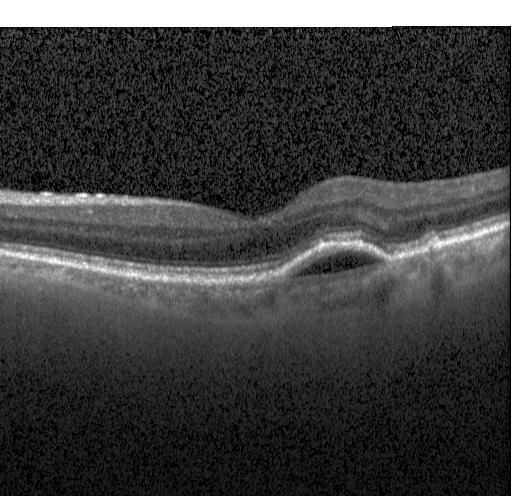 Through the macula; OCT line scan — Impression: choroidal neovascularization.